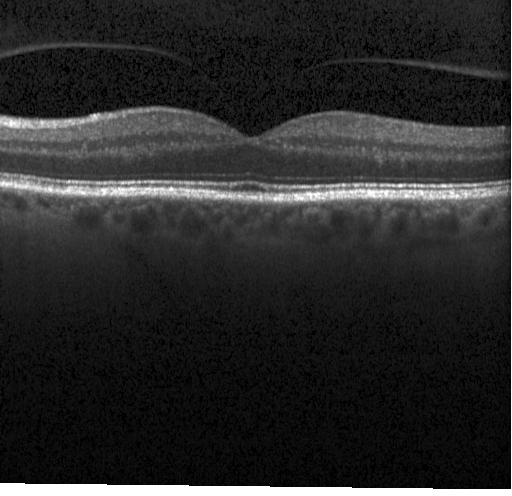 Acquired on a Heidelberg Spectralis · horizontal scan through the fovea · optical coherence tomography B-scan.
Impression: neither choroidal neovascularization, diabetic macular edema, nor drusen.